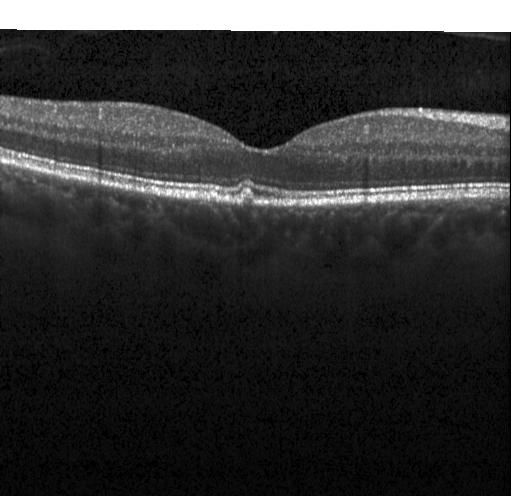

This B-scan demonstrates drusen.